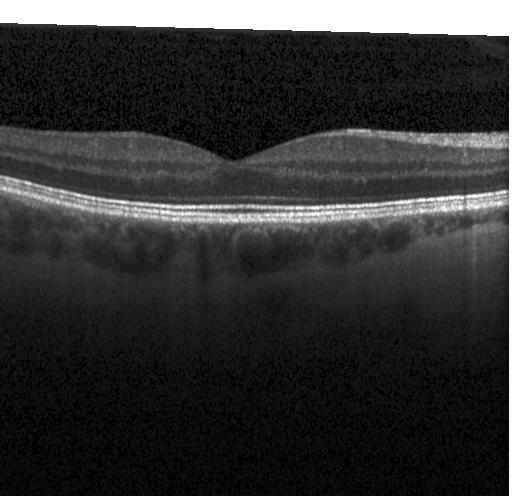
Spectral-domain OCT B-scan: no choroidal neovascularization, diabetic macular edema, or drusen.